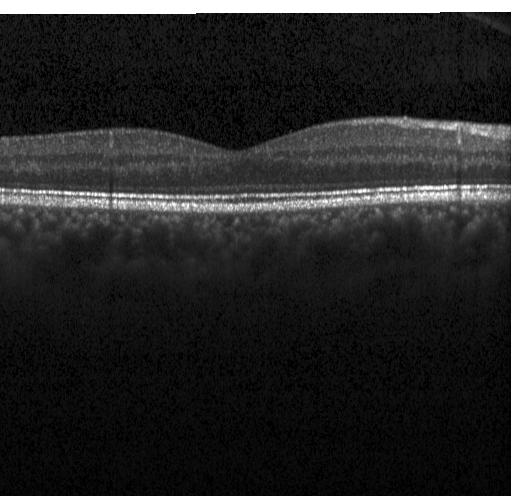 Spectral-domain OCT B-scan: no choroidal neovascularization, diabetic macular edema, or drusen.